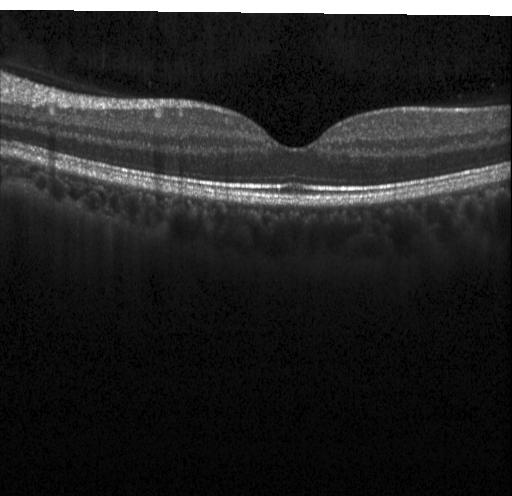 Spectral-domain optical coherence tomography; retinal OCT cross-section; centered on the fovea; Heidelberg Spectralis OCT system — Impression: no CNV, DME, or drusen.